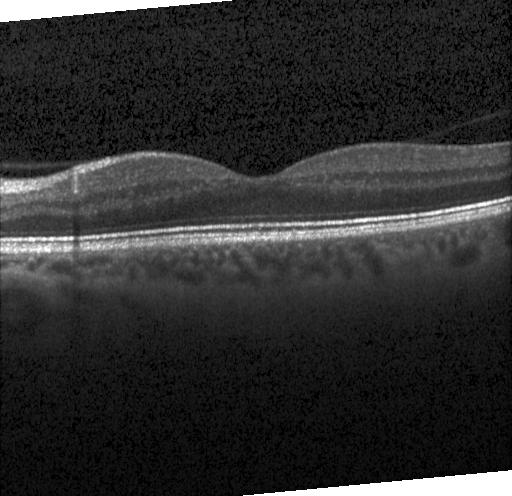 Retinal OCT B-scan; spectral-domain OCT — Diagnosis: neither choroidal neovascularization, diabetic macular edema, nor drusen.